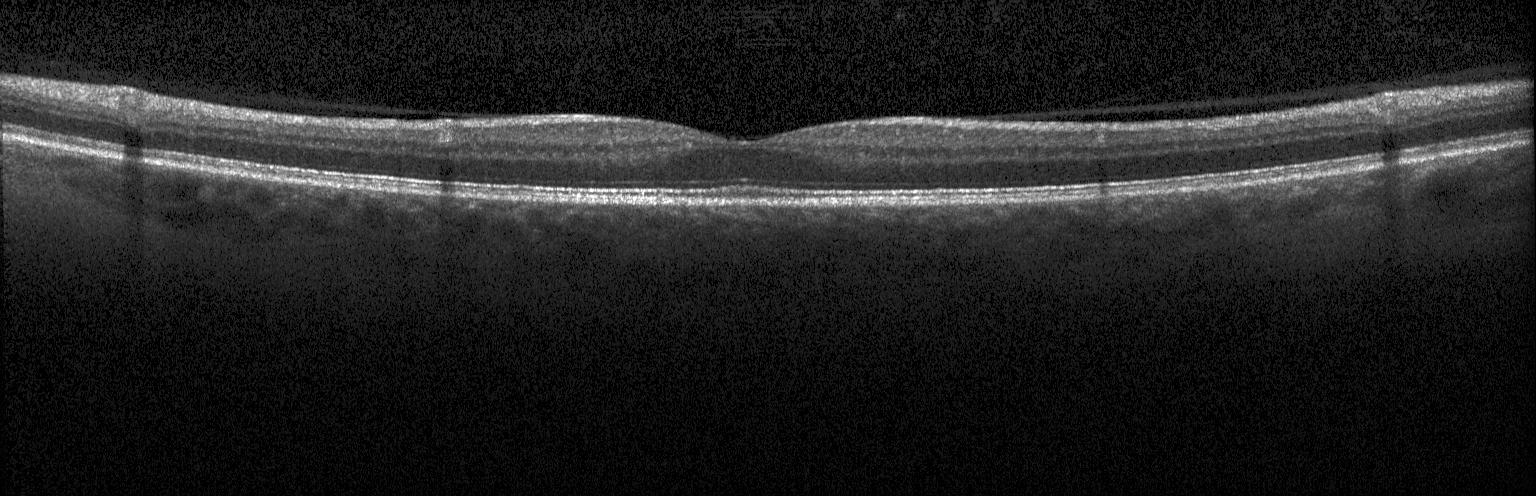 Retinal OCT B-scan. No choroidal neovascularization, diabetic macular edema, or drusen.